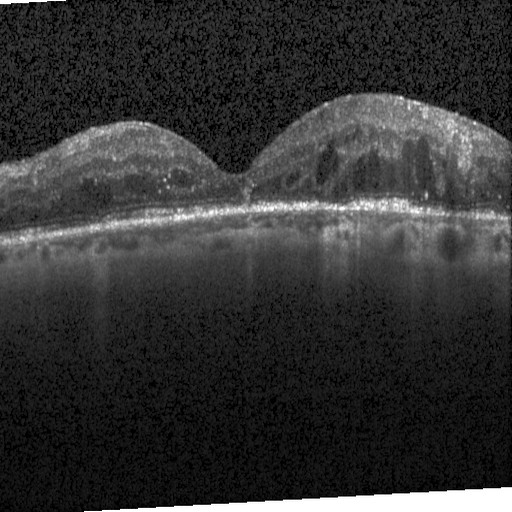
SD-OCT · through the macula · Heidelberg Spectralis OCT system · OCT B-scan
OCT finding: DME.